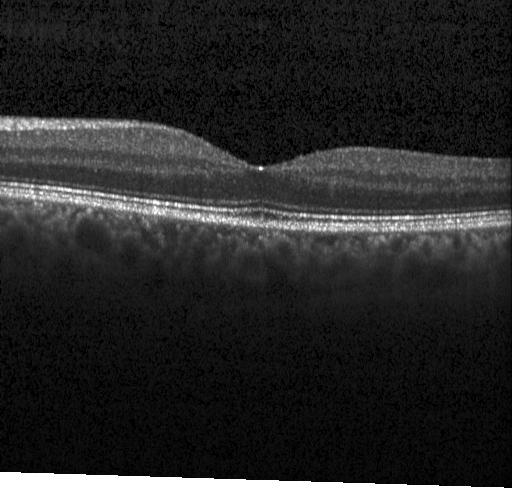 Optical coherence tomography B-scan. Macular OCT: neither CNV, DME, nor drusen.